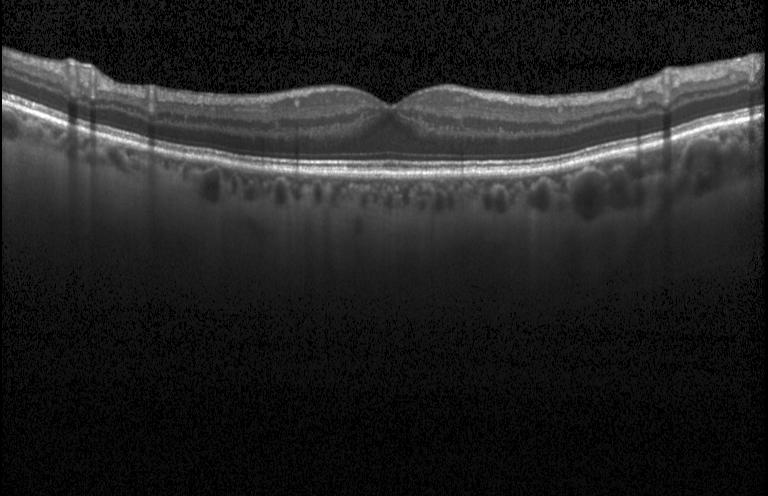
Macular OCT: no evidence of CNV, DME, or drusen.